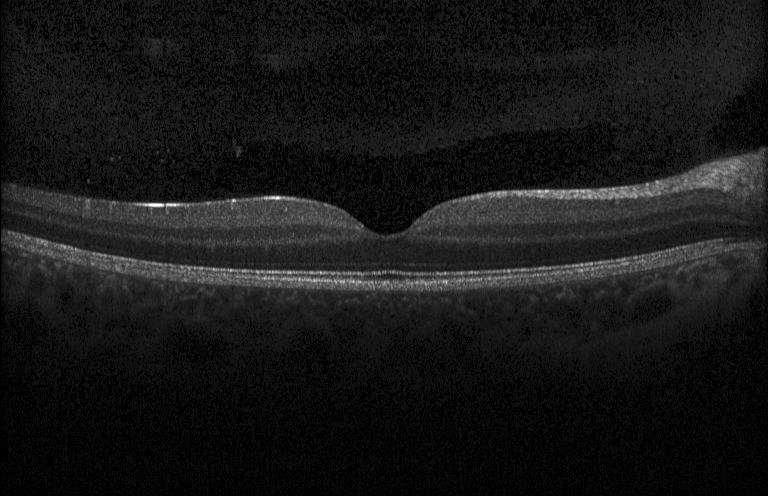 Finding: no choroidal neovascularization, diabetic macular edema, or drusen.